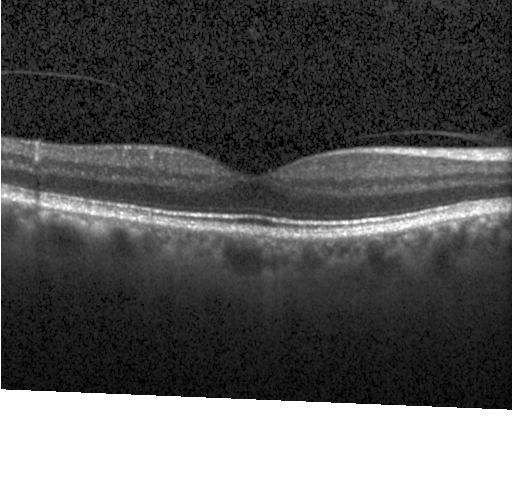
Optical coherence tomography scan.
Finding: no choroidal neovascularization, diabetic macular edema, or drusen.